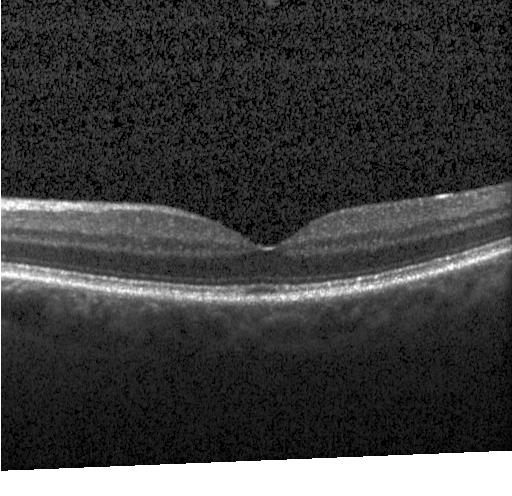
The scan shows no evidence of choroidal neovascularization, diabetic macular edema, or drusen.